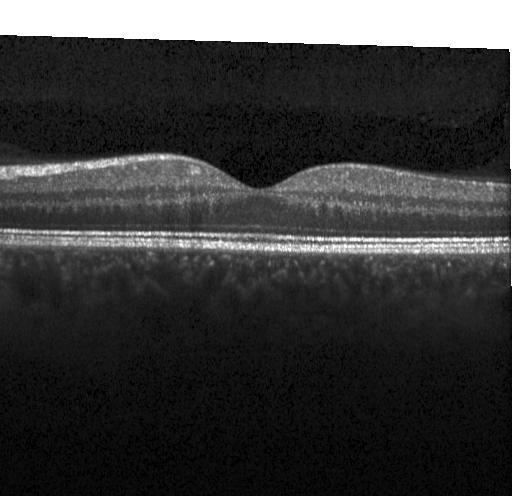
SD-OCT; optical coherence tomography B-scan; horizontal scan through the fovea; Heidelberg Spectralis — Diagnosis: no choroidal neovascularization, diabetic macular edema, or drusen.